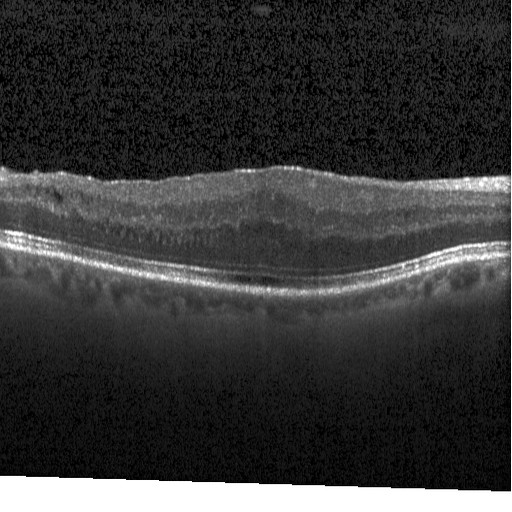

Finding: DME.